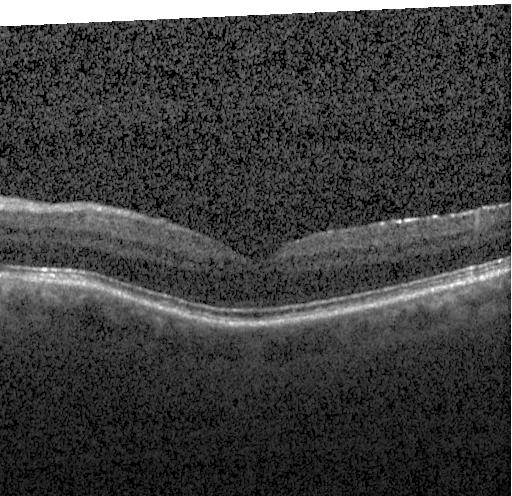

OCT scan showing no choroidal neovascularization, diabetic macular edema, or drusen.